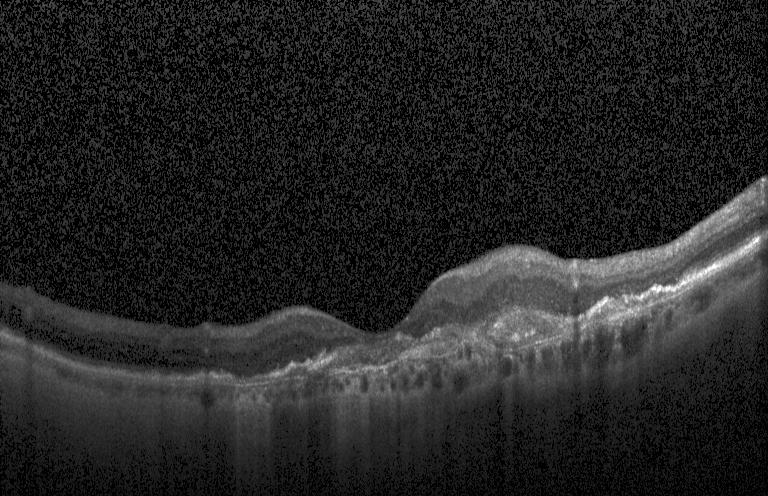 OCT B-scan — Finding: CNV.